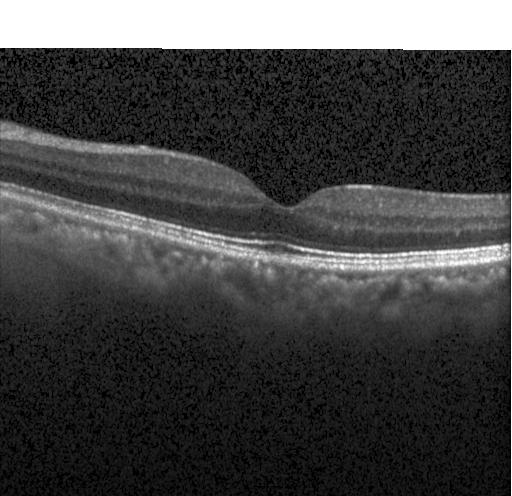 Macular scan, optical coherence tomography scan, instrument: Heidelberg Spectralis. Dx: no evidence of choroidal neovascularization, diabetic macular edema, or drusen.